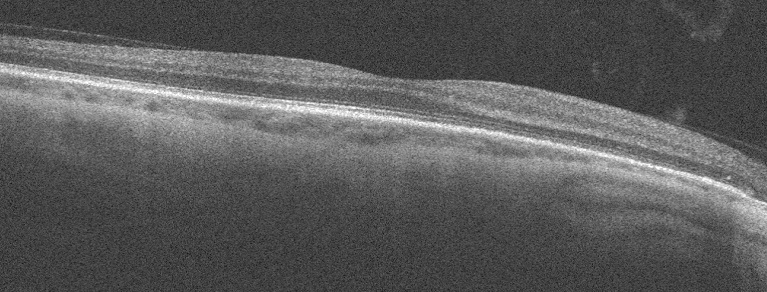

No AMD, DME, ERM, RAO, RVO, or VID.